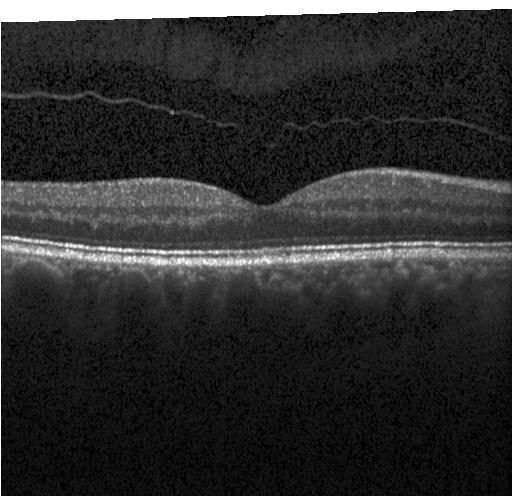

OCT scan showing no choroidal neovascularization, no diabetic macular edema, and no drusen.